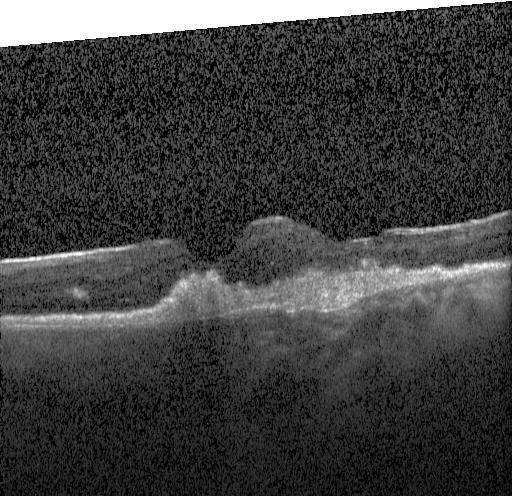
Heidelberg Spectralis OCT system; optical coherence tomography B-scan; spectral-domain optical coherence tomography
Choroidal neovascularization (CNV).